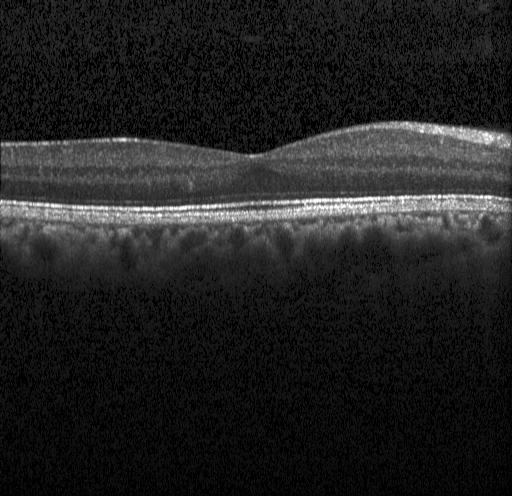
Through the macula, spectral-domain optical coherence tomography, acquired on a Heidelberg Spectralis, retinal OCT B-scan — Macular OCT: neither choroidal neovascularization, diabetic macular edema, nor drusen.